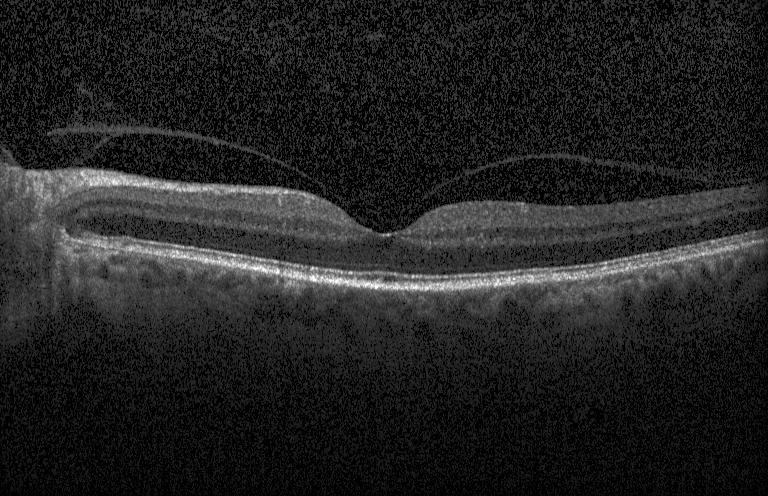 Finding: no evidence of choroidal neovascularization, diabetic macular edema, or drusen.